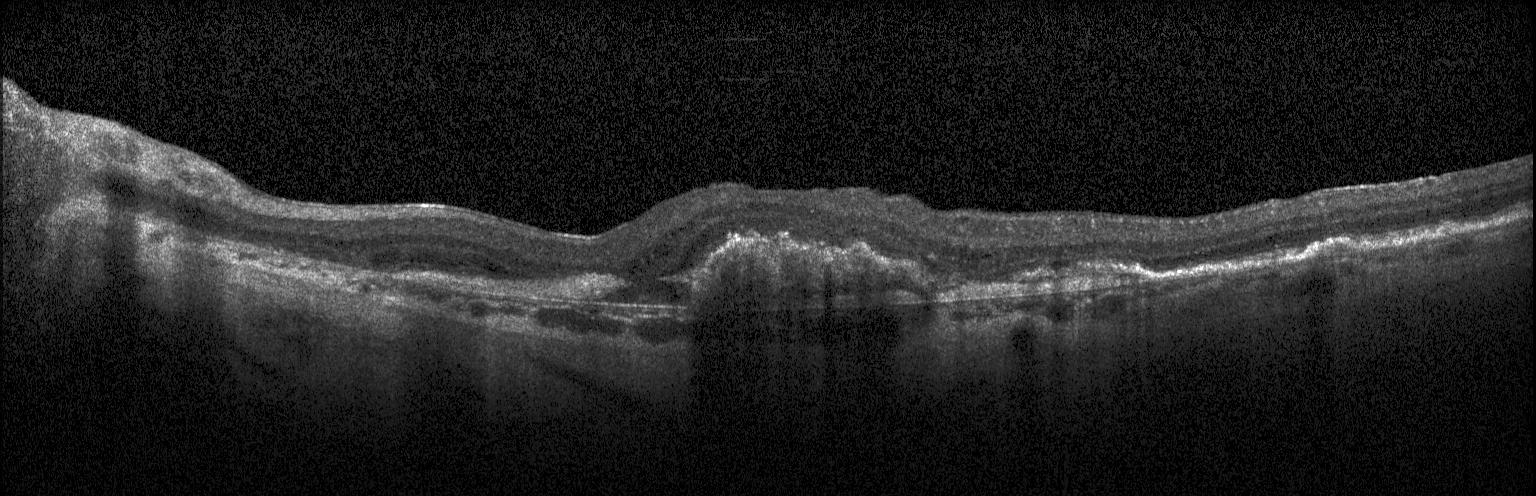
OCT B-scan; spectral-domain optical coherence tomography.
Assessment: a choroidal neovascular membrane.